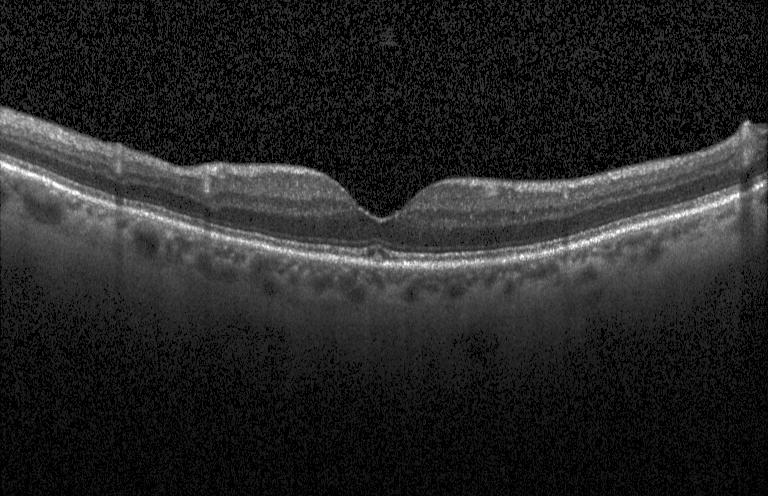
Retinal OCT B-scan · spectral-domain optical coherence tomography.
Neither CNV, DME, nor drusen.